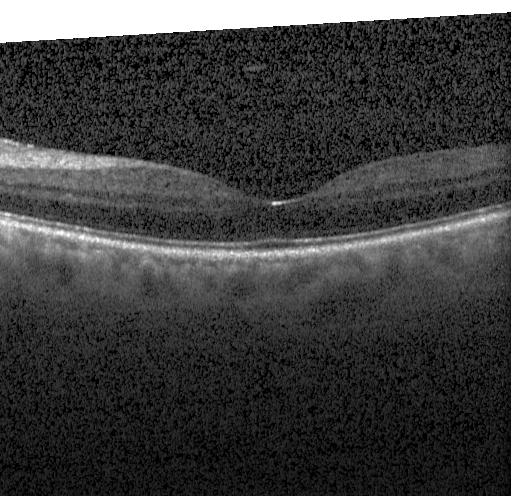
OCT line scan.
Impression: neither choroidal neovascularization, diabetic macular edema, nor drusen.